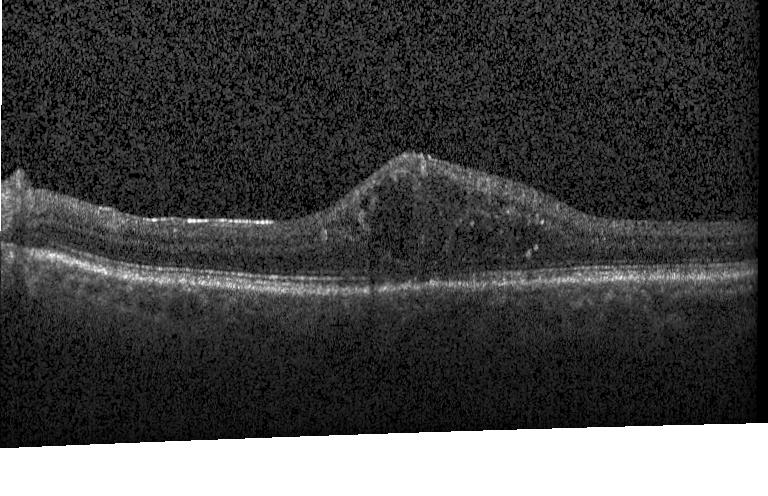
Optical coherence tomography B-scan; acquired on a Heidelberg Spectralis; horizontal scan through the fovea
OCT finding: diabetic macular edema.